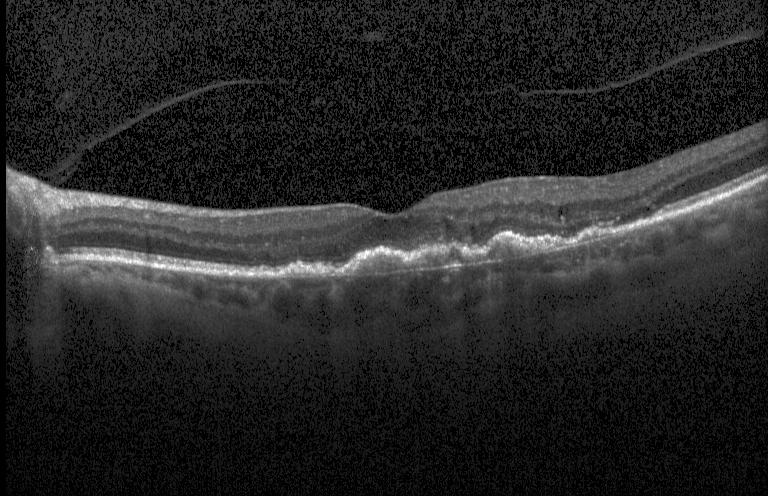

A choroidal neovascular membrane.